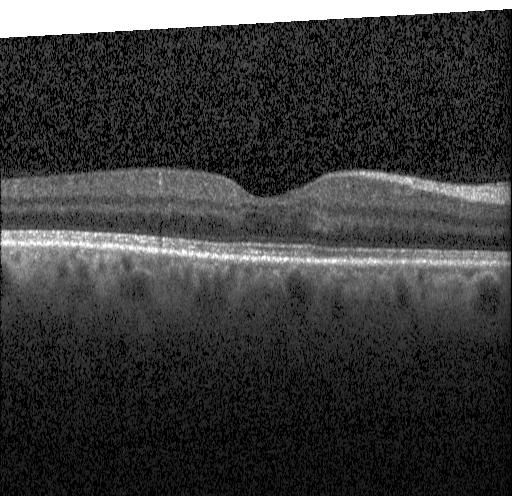

Macular OCT demonstrating neither CNV, DME, nor drusen.